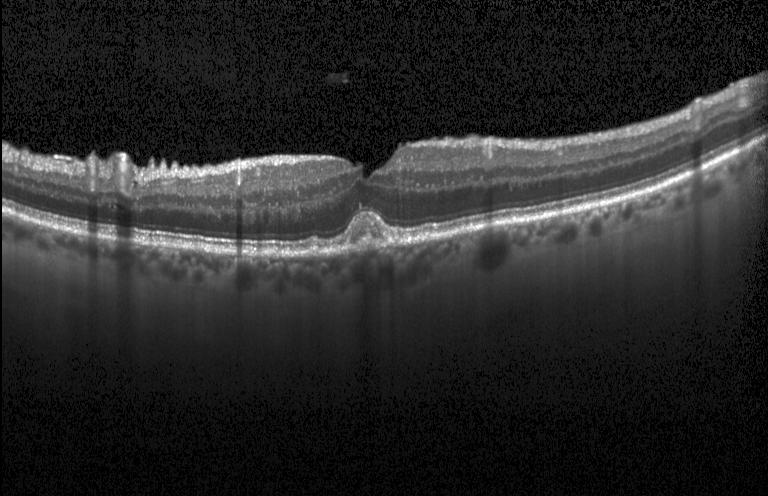

Spectral-domain OCT · Heidelberg Spectralis · retinal OCT cross-section
Assessment: sub-RPE drusenoid deposits.